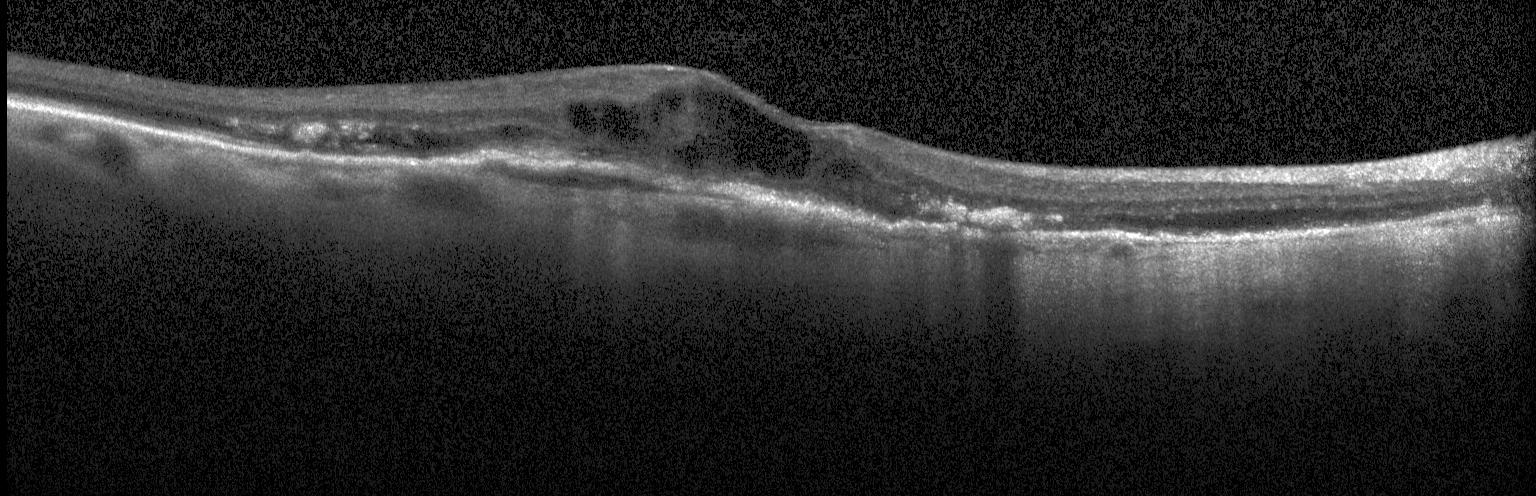
Macular OCT: a choroidal neovascular membrane.